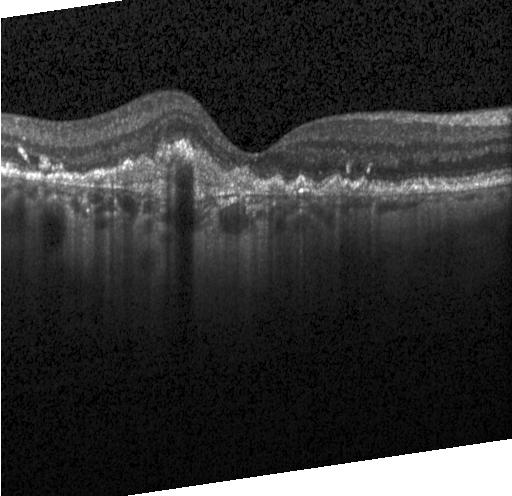 This B-scan demonstrates a choroidal neovascular membrane.